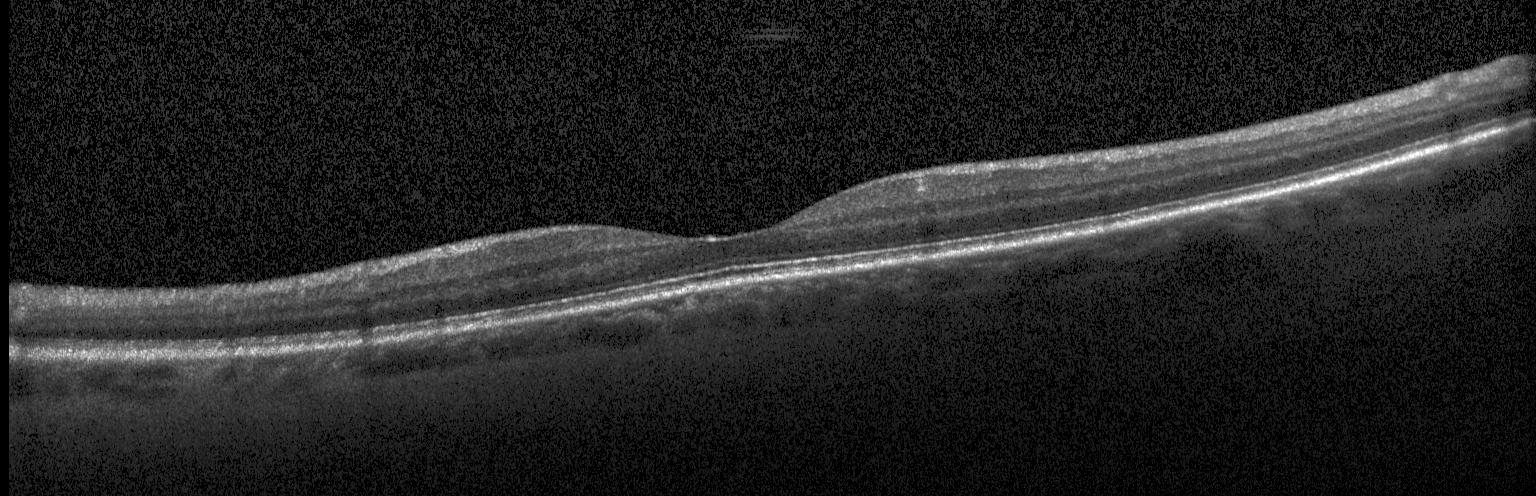

The scan shows no choroidal neovascularization, diabetic macular edema, or drusen.